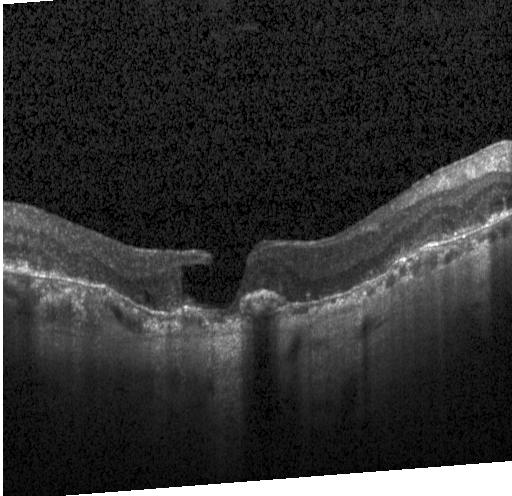 Instrument: Heidelberg Spectralis; spectral-domain optical coherence tomography; retinal OCT B-scan — Macular OCT: choroidal neovascularization (CNV).